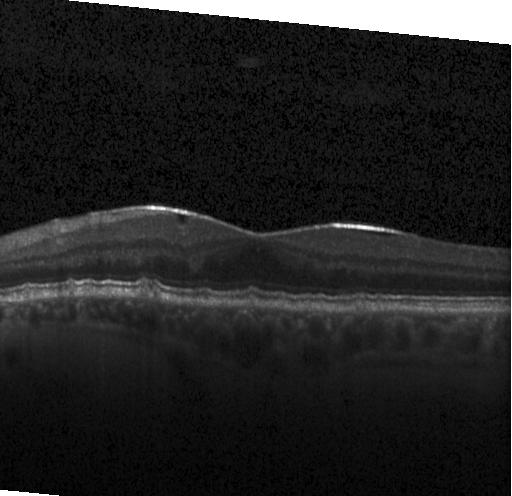
Optical coherence tomography B-scan — Macular OCT: multiple drusen.